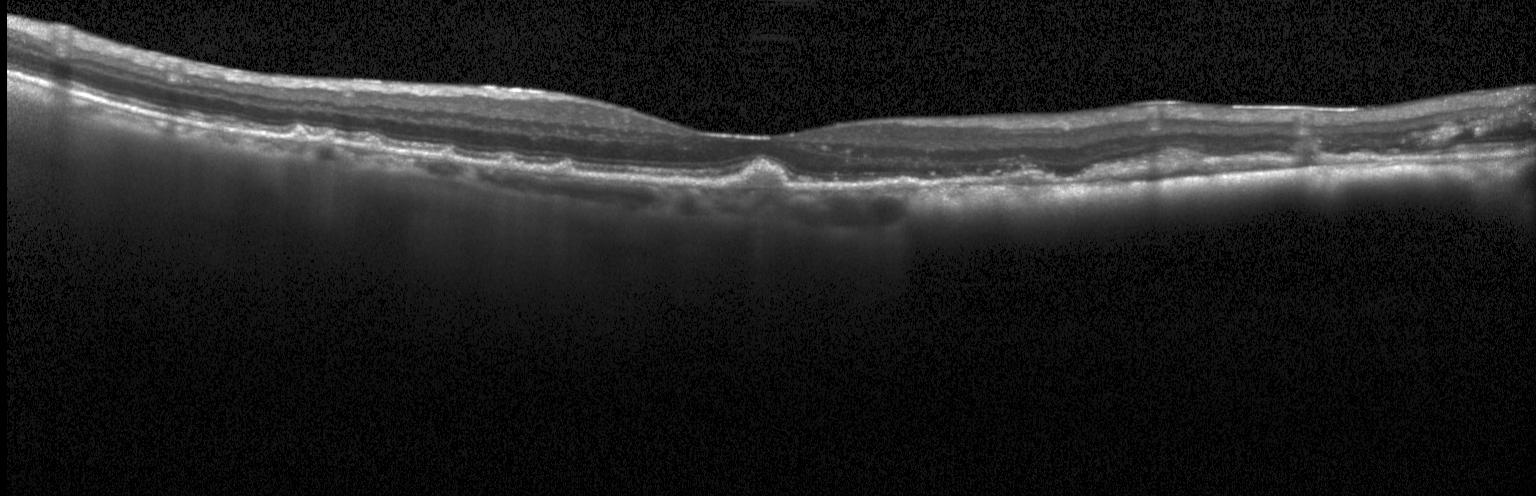
Macular OCT: a choroidal neovascular membrane.